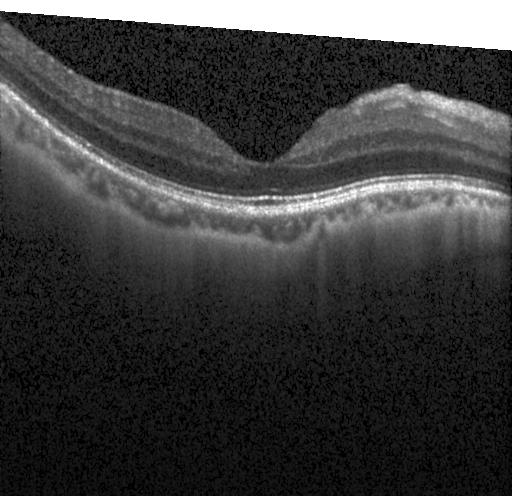 Spectral-domain OCT B-scan: neither choroidal neovascularization, diabetic macular edema, nor drusen.